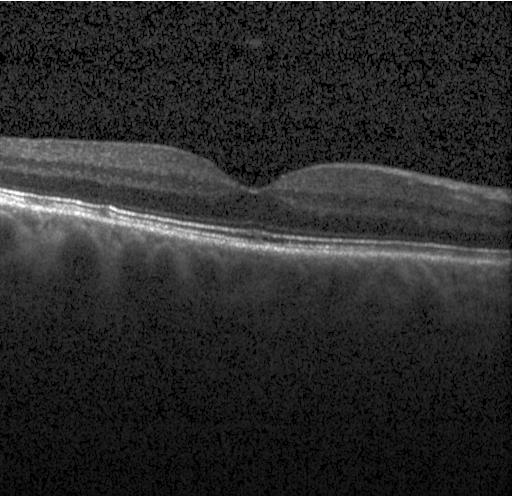

Spectral-domain OCT. Optical coherence tomography scan. Fovea-centered. Finding: no choroidal neovascularization, no diabetic macular edema, and no drusen.